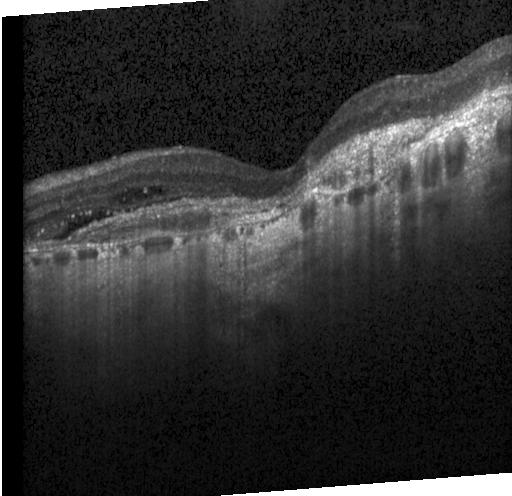 Impression: a choroidal neovascular membrane.